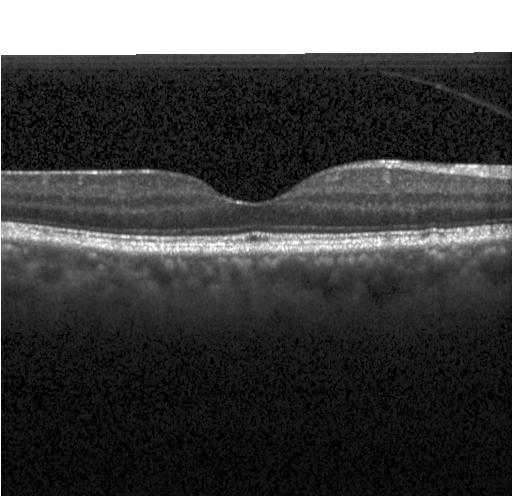 Optical coherence tomography B-scan · acquired on a Heidelberg Spectralis · spectral-domain OCT.
Impression: no evidence of CNV, DME, or drusen.